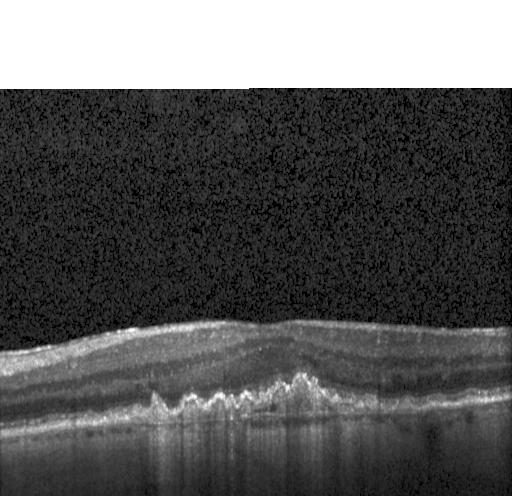 Retinal OCT cross-section showing choroidal neovascularization.